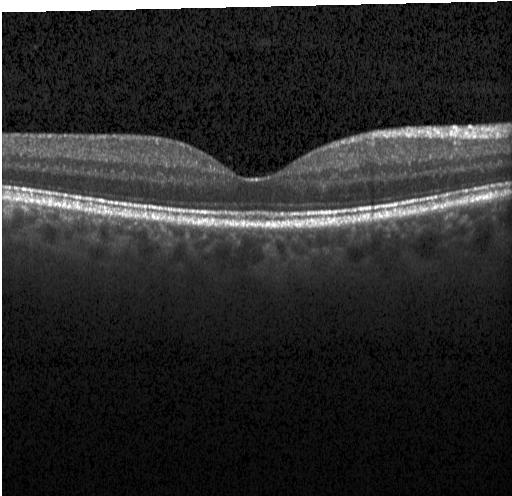

Retinal OCT B-scan; SD-OCT — Macular OCT: neither choroidal neovascularization, diabetic macular edema, nor drusen.